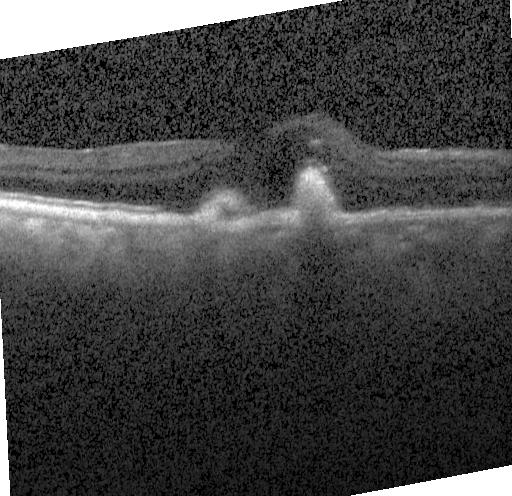 Impression: choroidal neovascularization (CNV).